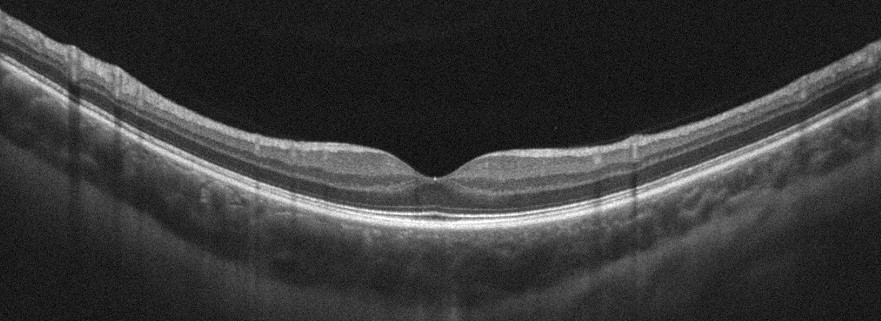
Acquired on an Optovue Avanti RTVue XR, optical coherence tomography scan. Diagnosis: absence of AMD, DME, ERM, RAO, RVO, and vitreomacular interface disease.